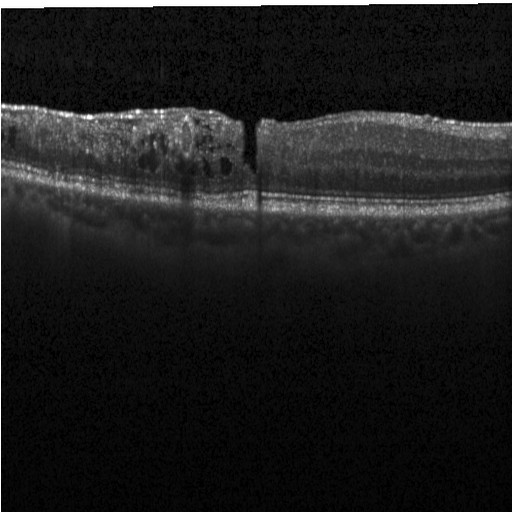
DME.